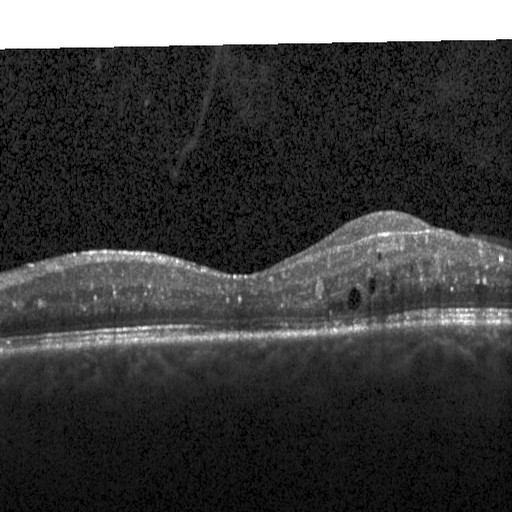

Assessment: diabetic macular edema (DME).